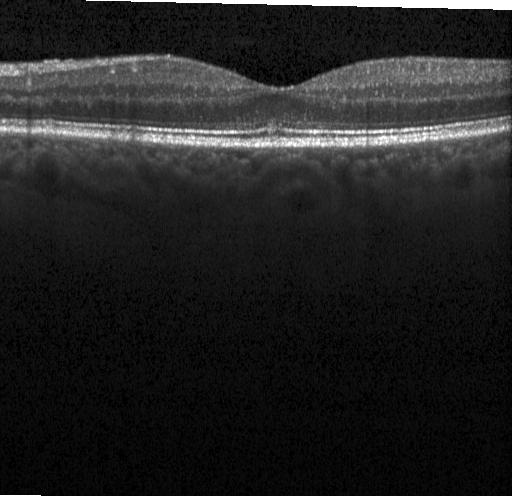
OCT scan showing no choroidal neovascularization, diabetic macular edema, or drusen.